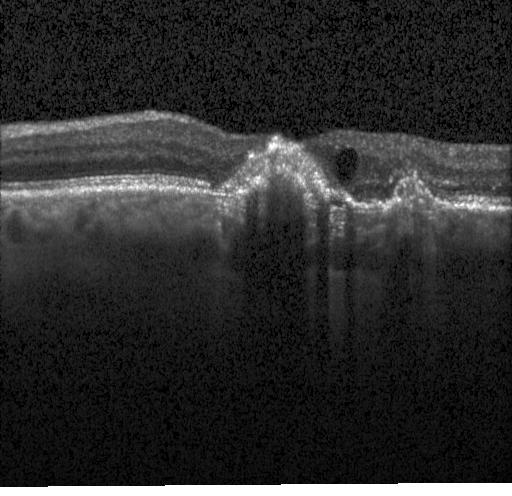 Heidelberg Spectralis. Centered on the fovea. Optical coherence tomography B-scan. Spectral-domain OCT. Impression: choroidal neovascularization.